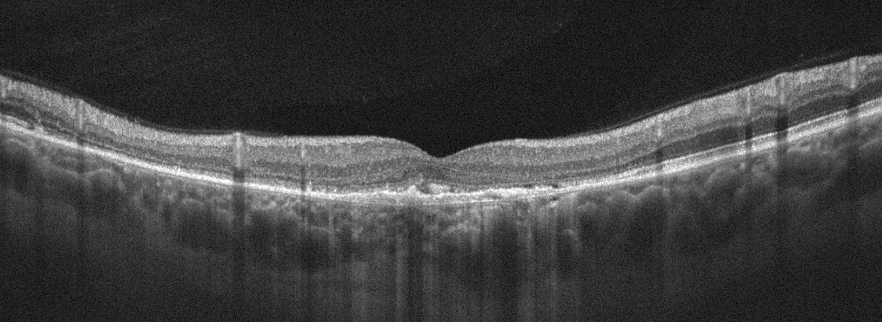 Retinal OCT B-scan; right eye.
Finding: age-related macular degeneration.